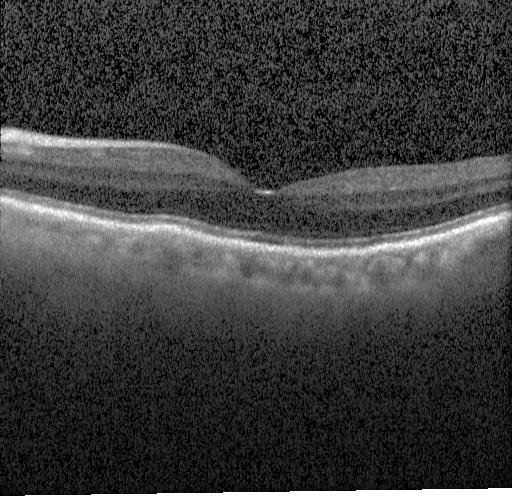 Optical coherence tomography scan. Horizontal scan through the fovea. Instrument: Heidelberg Spectralis.
Finding: no choroidal neovascularization, diabetic macular edema, or drusen.